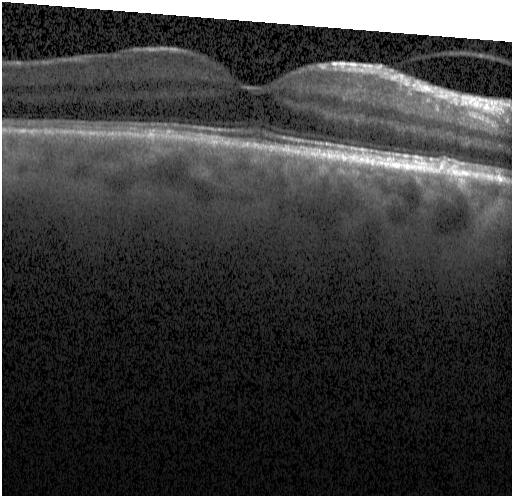

OCT B-scan; spectral-domain OCT
Diagnosis: no choroidal neovascularization, no diabetic macular edema, and no drusen.